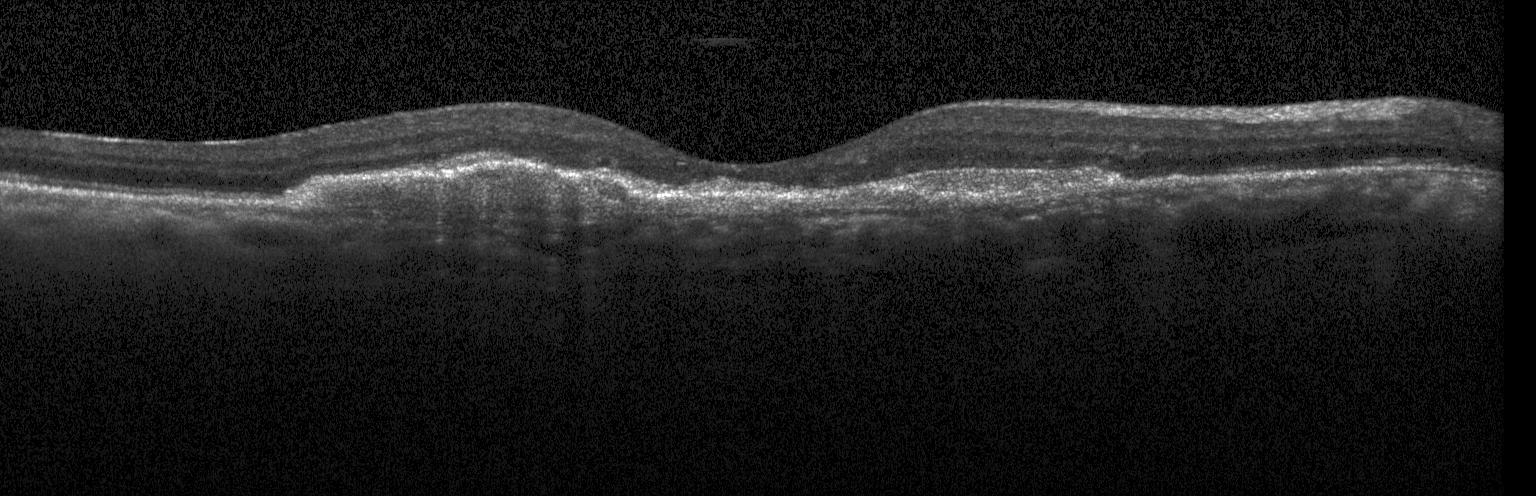 Optical coherence tomography B-scan.
The scan shows choroidal neovascularization (CNV).